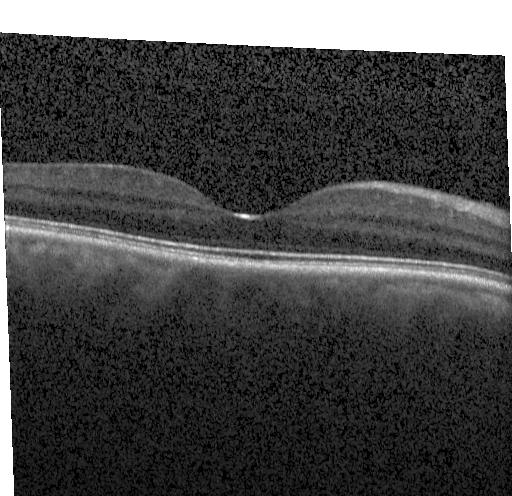
Heidelberg Spectralis OCT system; OCT B-scan; SD-OCT; fovea-centered
Impression: neither choroidal neovascularization, diabetic macular edema, nor drusen.